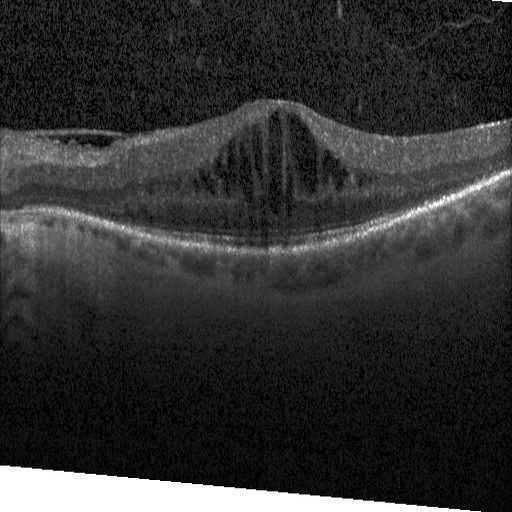
Retinal OCT cross-section. Impression: DME.